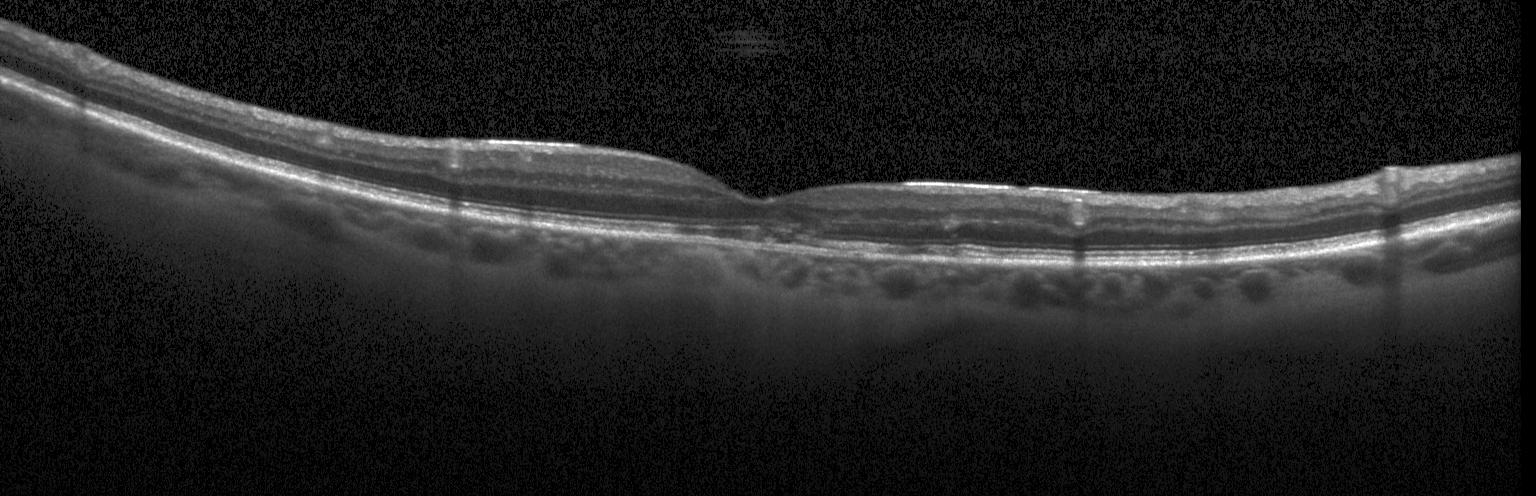 Diagnosis: a choroidal neovascular membrane.